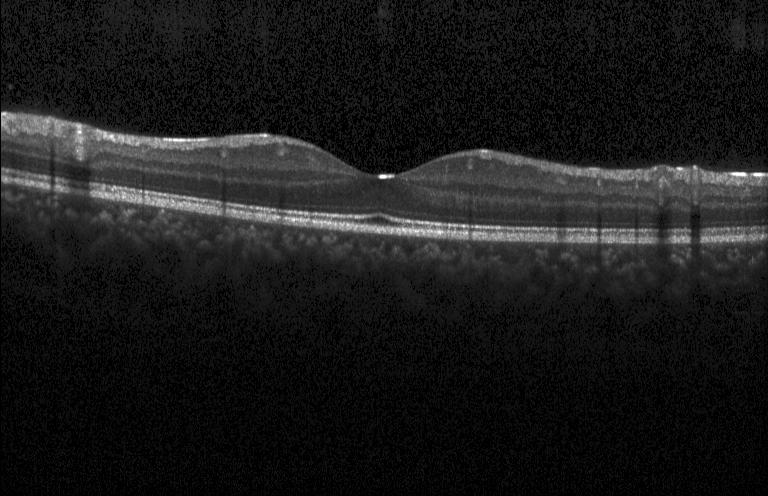 Instrument: Heidelberg Spectralis; through the macula; SD-OCT; optical coherence tomography B-scan — Diagnosis: neither CNV, DME, nor drusen.